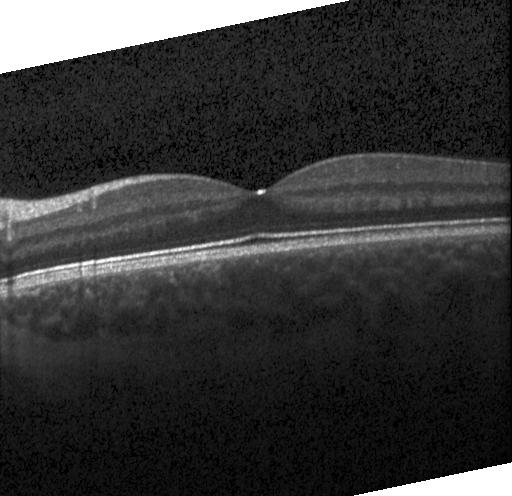

Retinal OCT cross-section. Assessment: neither CNV, DME, nor drusen.